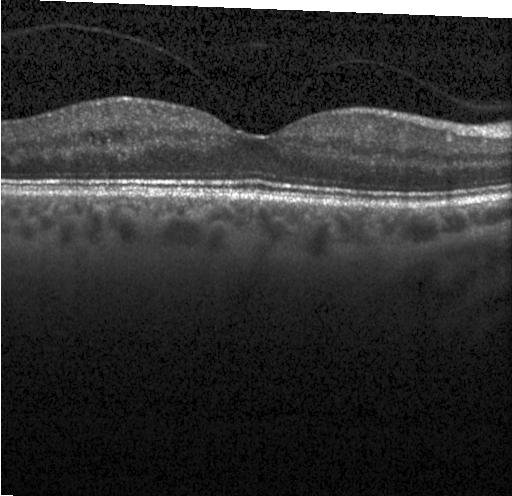

Heidelberg Spectralis. OCT line scan — Diabetic macular edema.